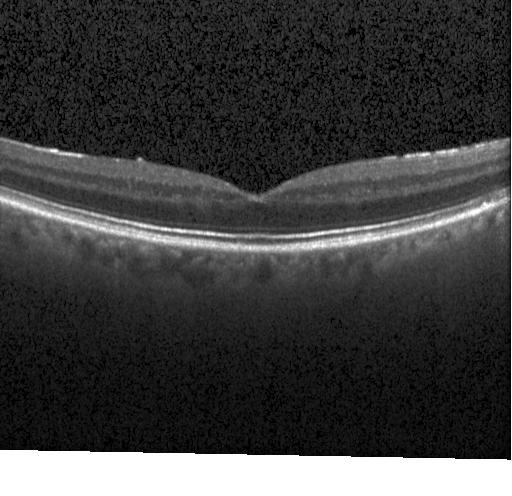 OCT B-scan. Horizontal scan through the fovea. Instrument: Heidelberg Spectralis. The scan shows no evidence of choroidal neovascularization, diabetic macular edema, or drusen.